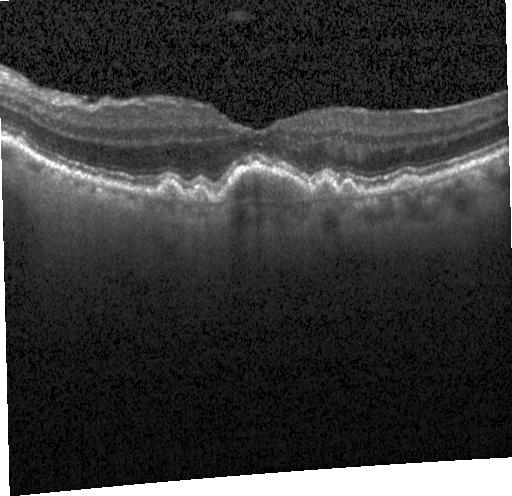

OCT B-scan
Finding: CNV.